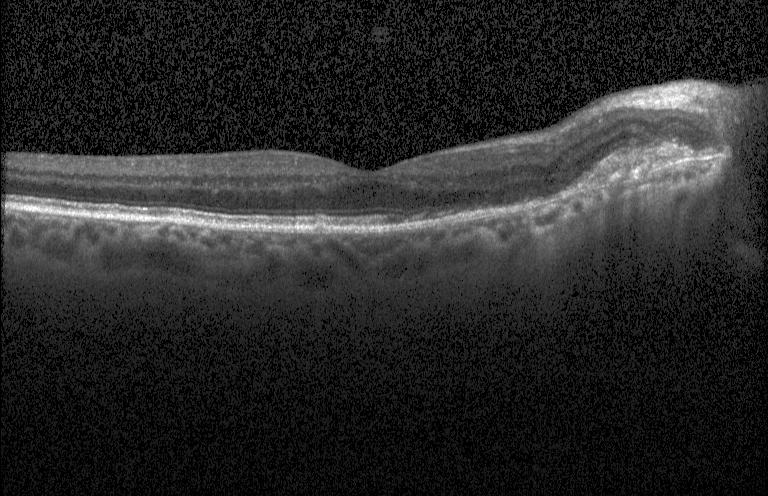
Retinal OCT B-scan; acquired on a Heidelberg Spectralis; SD-OCT. Diagnosis: a choroidal neovascular membrane.